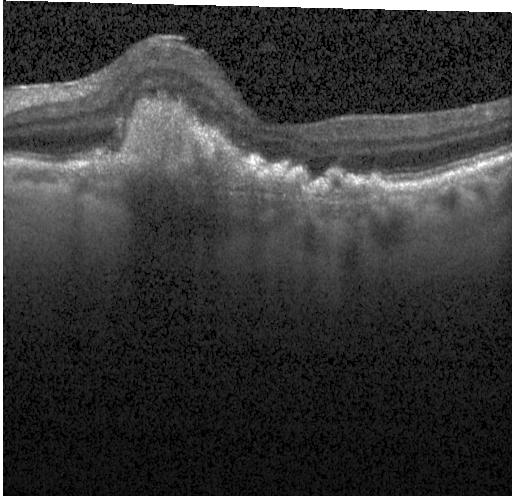

Retinal OCT cross-section showing choroidal neovascularization.